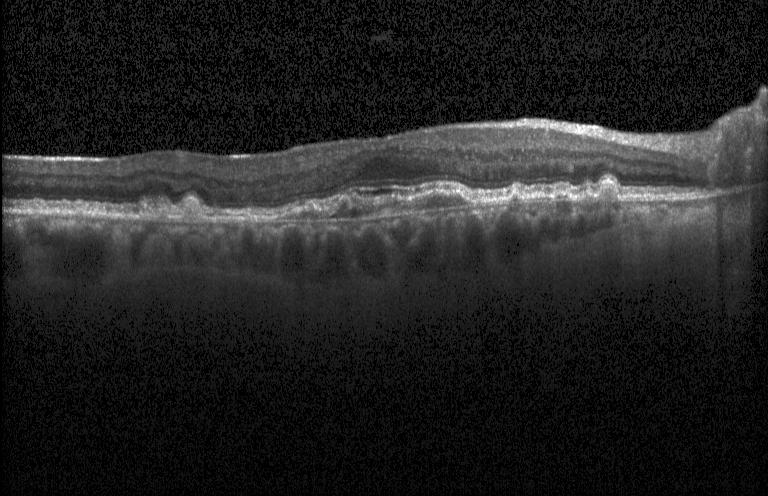 Diagnosis: a choroidal neovascular membrane.